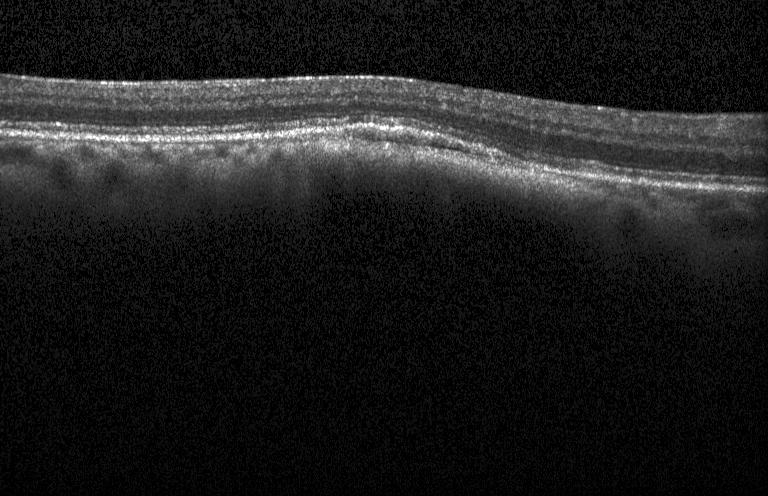

Finding: a choroidal neovascular membrane.